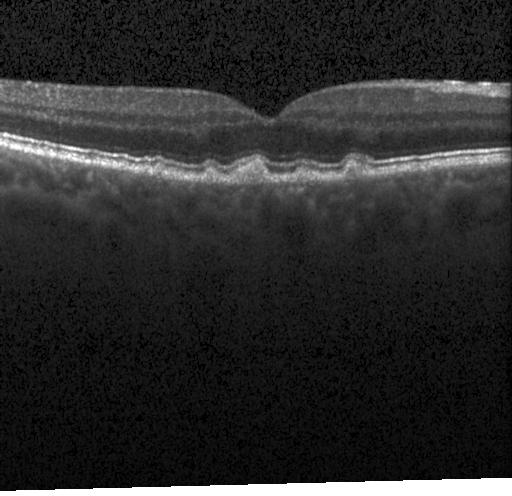 Optical coherence tomography scan
Drusen.